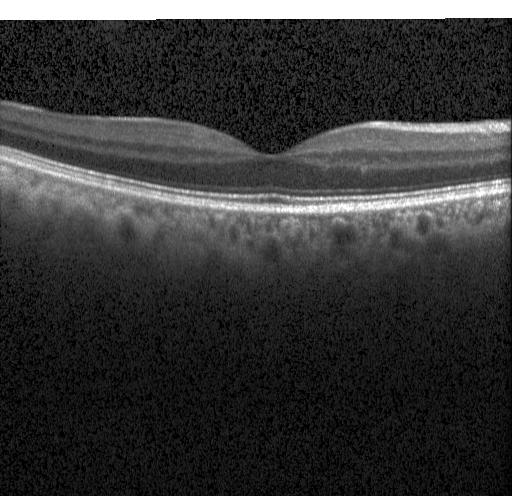

Heidelberg Spectralis OCT system · SD-OCT · optical coherence tomography scan · fovea-centered — The scan shows neither choroidal neovascularization, diabetic macular edema, nor drusen.